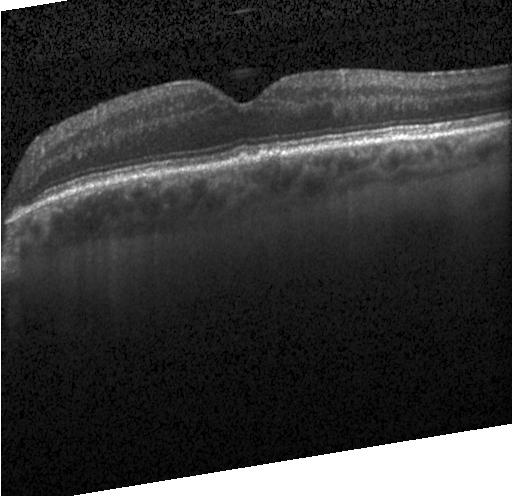

Macular scan. Retinal OCT B-scan. Sub-RPE drusenoid deposits.